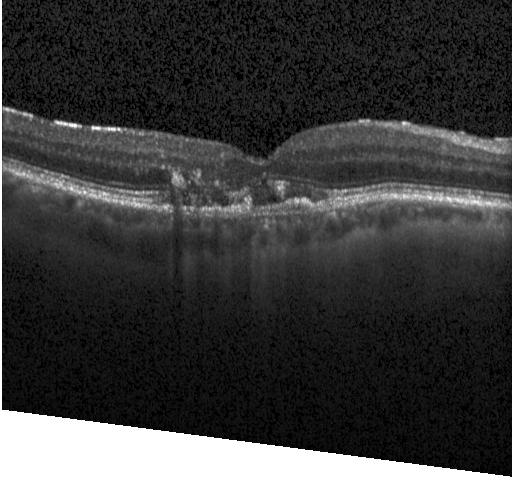 Impression: choroidal neovascularization (CNV).